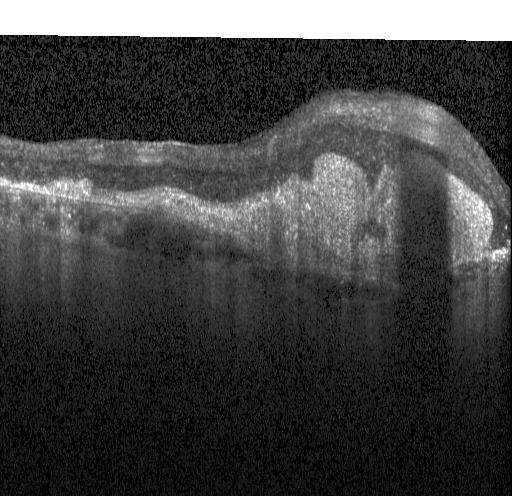
Diagnosis: a choroidal neovascular membrane.